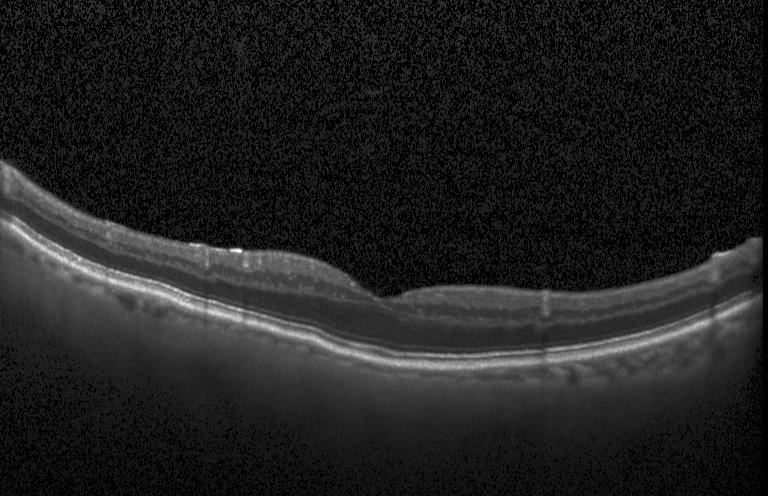 OCT finding: no evidence of choroidal neovascularization, diabetic macular edema, or drusen.